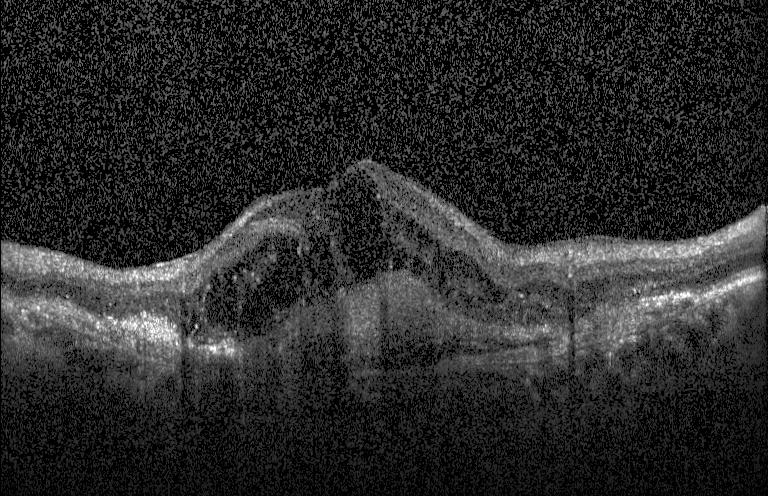

Fovea-centered. SD-OCT. Instrument: Heidelberg Spectralis. Retinal OCT B-scan. The scan shows a choroidal neovascular membrane.